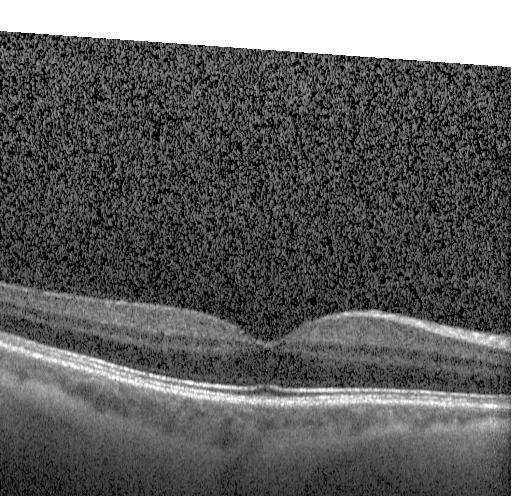
Spectral-domain optical coherence tomography. Optical coherence tomography B-scan. Through the macula.
Diagnosis: neither choroidal neovascularization, diabetic macular edema, nor drusen.